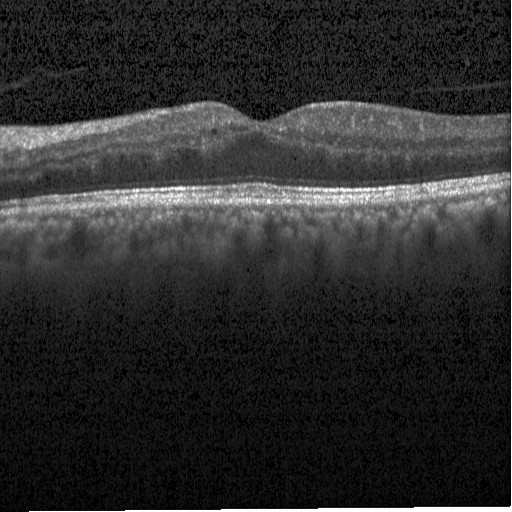
Assessment: diabetic macular edema.